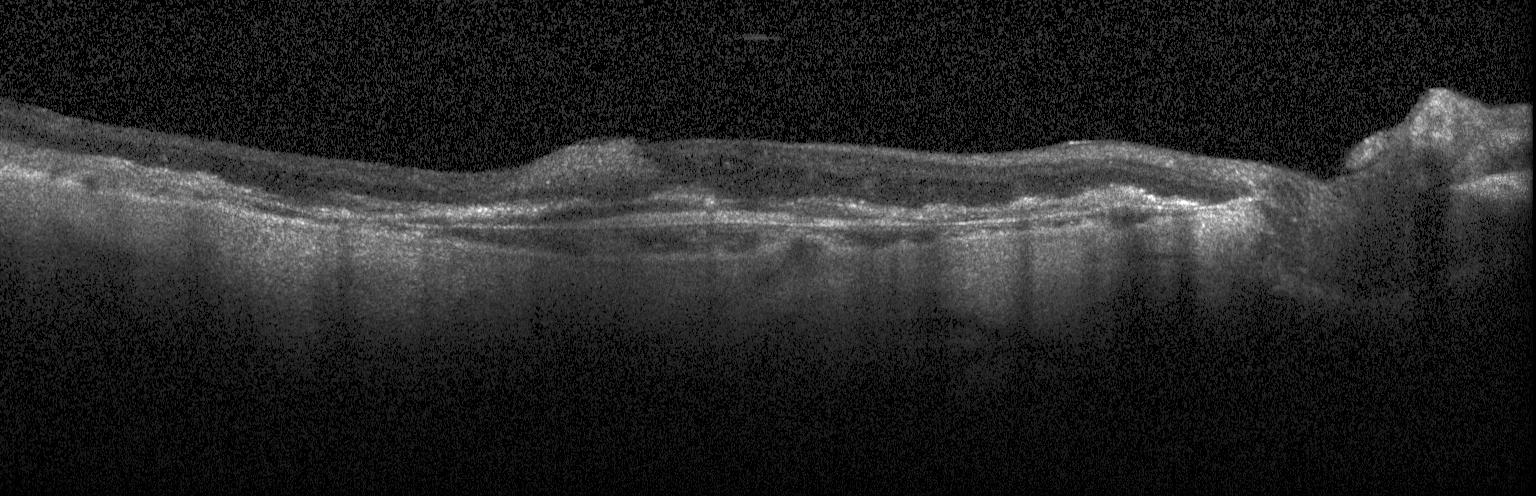 OCT B-scan. Fovea-centered. Heidelberg Spectralis. Assessment: a choroidal neovascular membrane.